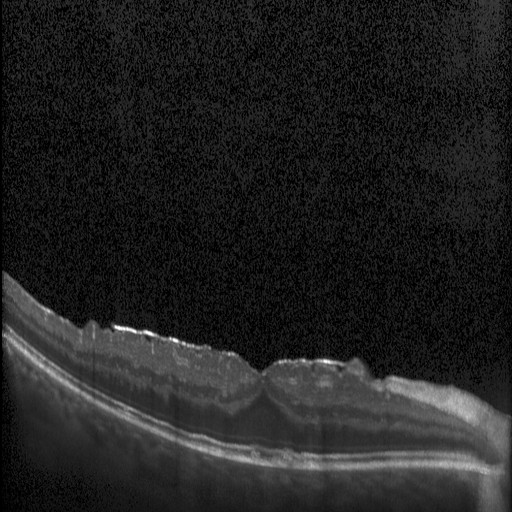 OCT B-scan · fovea-centered · SD-OCT. This B-scan demonstrates diabetic macular edema.